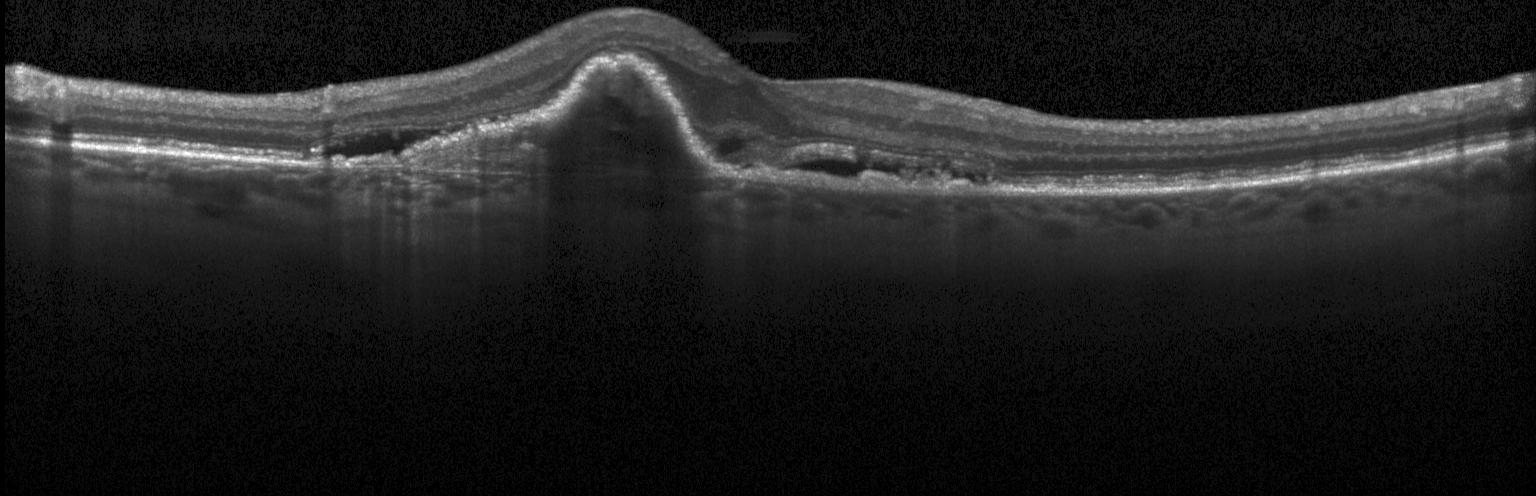
Finding: a choroidal neovascular membrane.